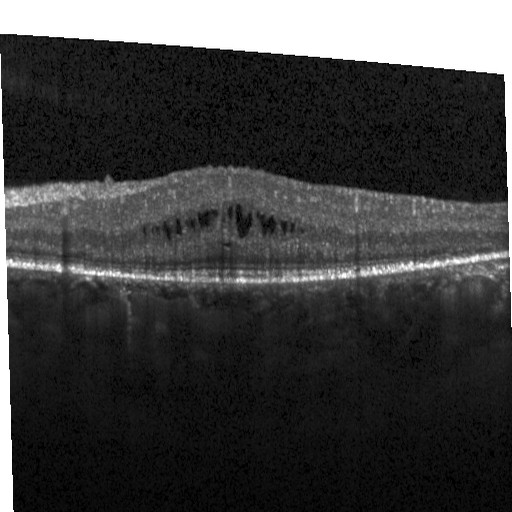

Optical coherence tomography scan. Heidelberg Spectralis OCT system — This B-scan demonstrates DME.